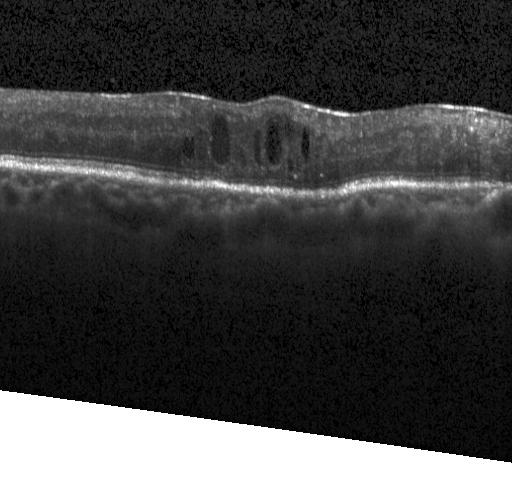

Acquired on a Heidelberg Spectralis; OCT B-scan; horizontal scan through the fovea; spectral-domain optical coherence tomography
Dx: diabetic macular edema.